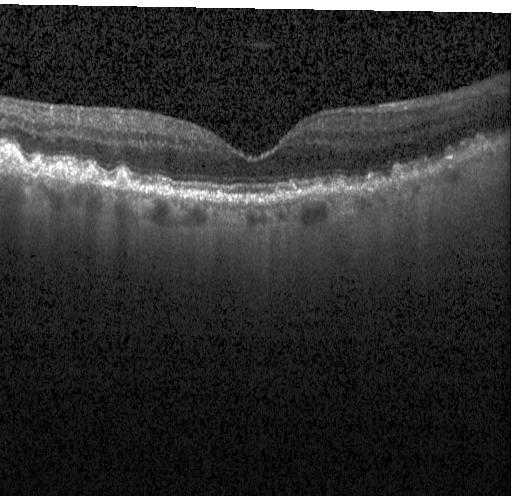
Macular scan, acquired on a Heidelberg Spectralis, OCT line scan, spectral-domain OCT. Dx: drusen.